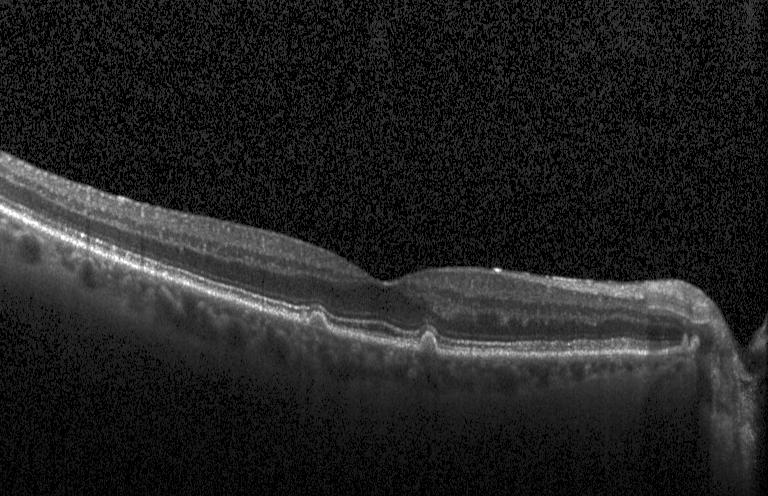 SD-OCT, retinal OCT cross-section, Heidelberg Spectralis. Sub-RPE drusenoid deposits.